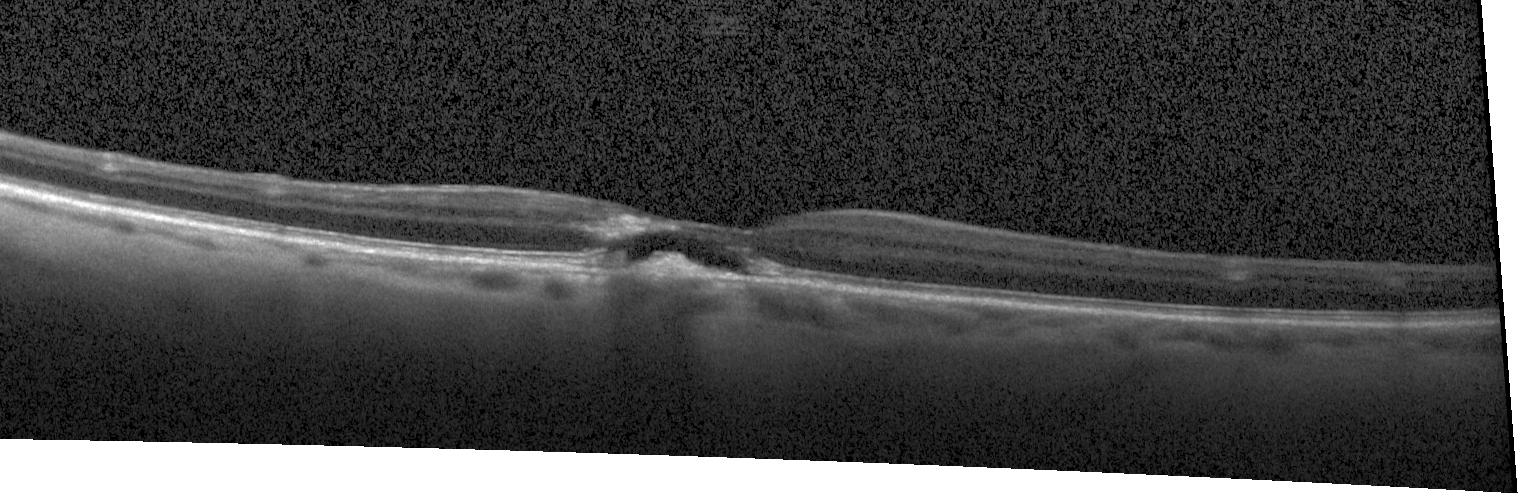
OCT B-scan showing a choroidal neovascular membrane.